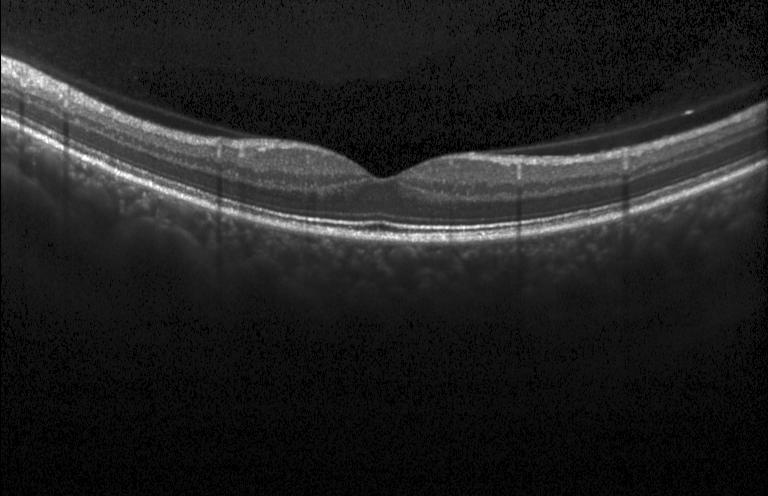
Impression: no choroidal neovascularization, no diabetic macular edema, and no drusen.